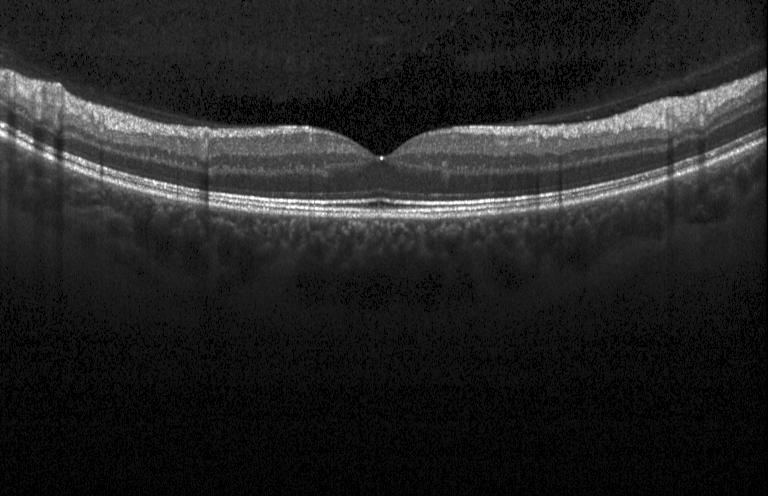
OCT line scan — Neither CNV, DME, nor drusen.